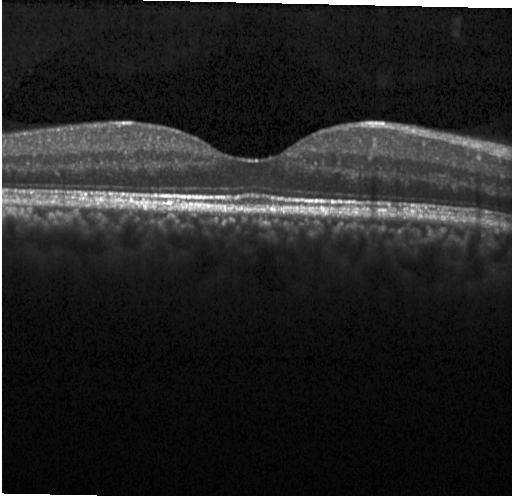
Optical coherence tomography scan; Heidelberg Spectralis
Assessment: no choroidal neovascularization, no diabetic macular edema, and no drusen.